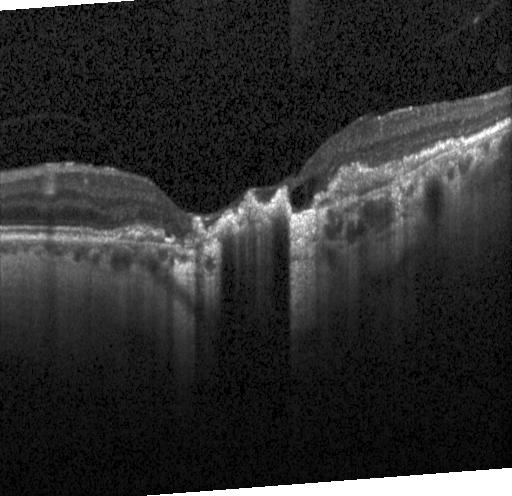
Through the macula. OCT B-scan. Spectral-domain OCT.
Impression: a choroidal neovascular membrane.